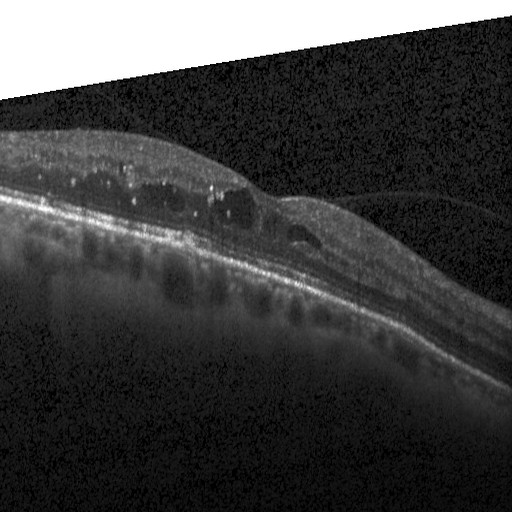 Macular scan, Heidelberg Spectralis OCT system, SD-OCT, OCT B-scan — Finding: diabetic macular edema (DME).